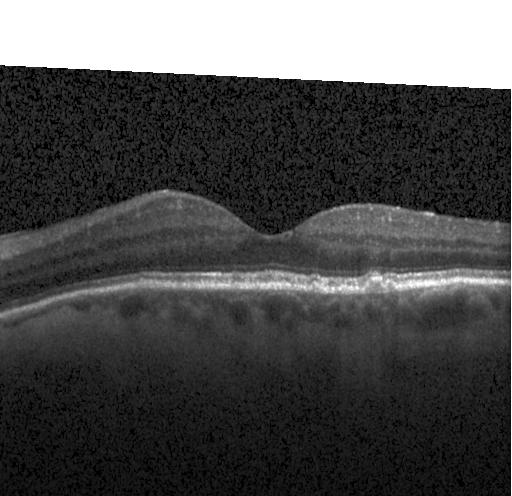 Assessment: multiple drusen.